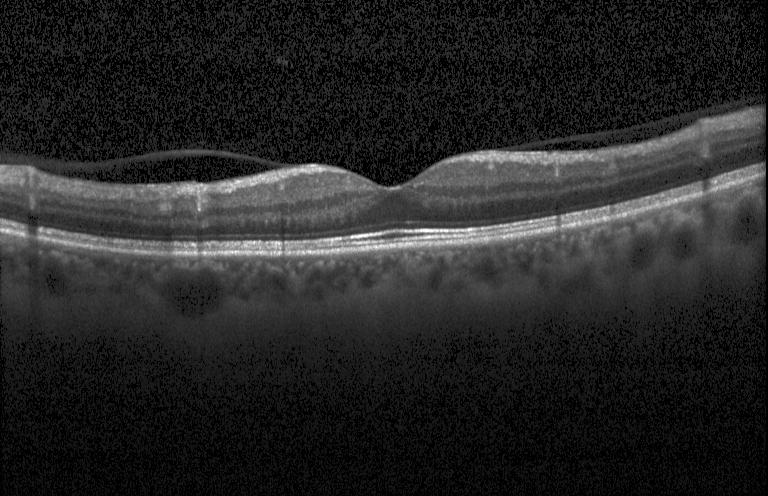
Impression: neither CNV, DME, nor drusen.